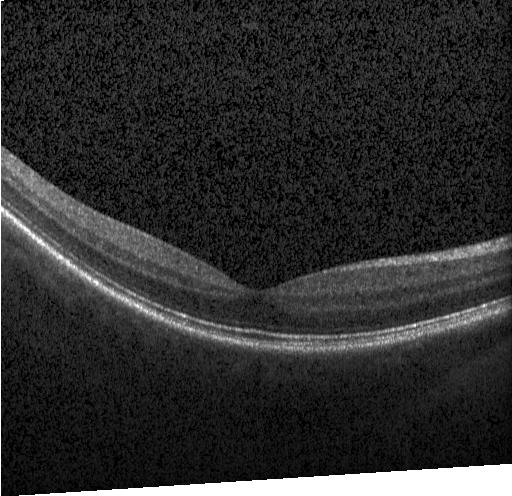 Fovea-centered; retinal OCT B-scan
This B-scan demonstrates neither CNV, DME, nor drusen.